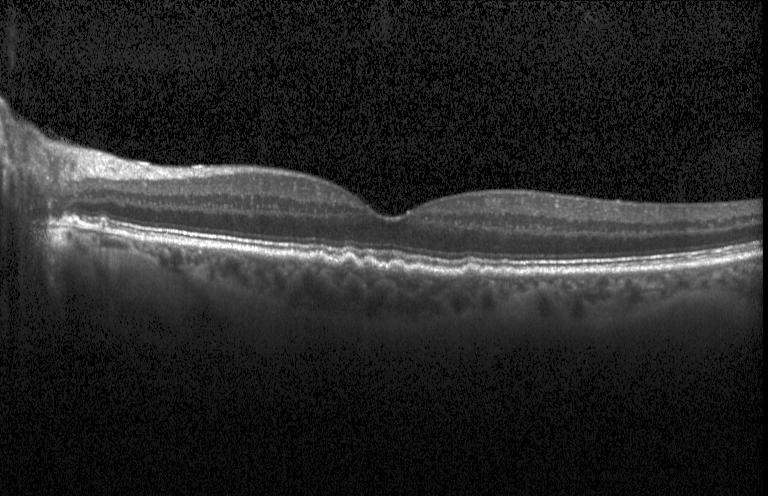 Multiple drusen.